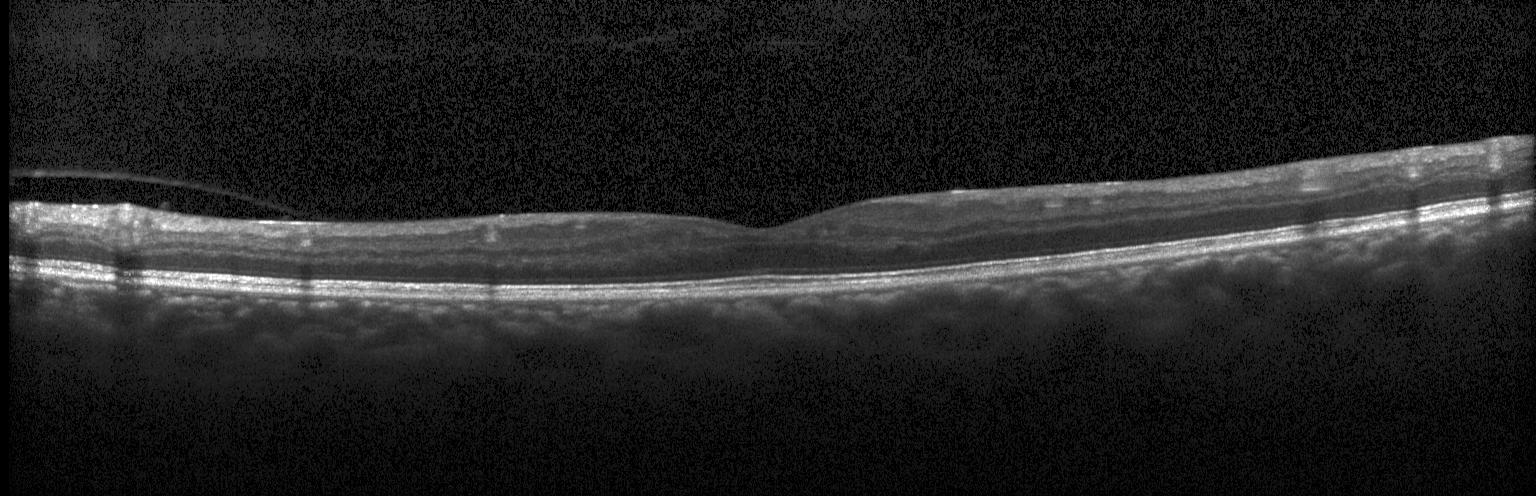
Retinal OCT cross-section — This B-scan demonstrates neither choroidal neovascularization, diabetic macular edema, nor drusen.